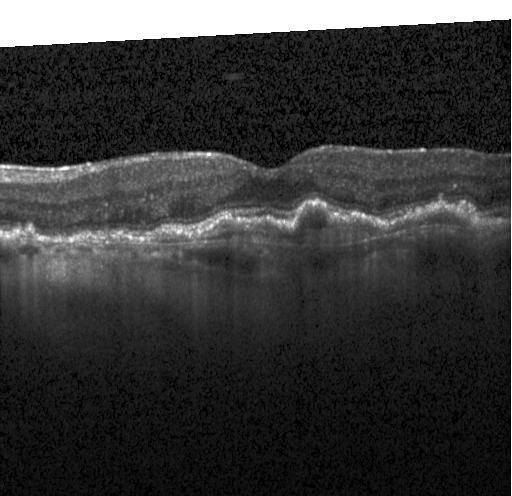 Optical coherence tomography scan, spectral-domain optical coherence tomography. Assessment: a choroidal neovascular membrane.